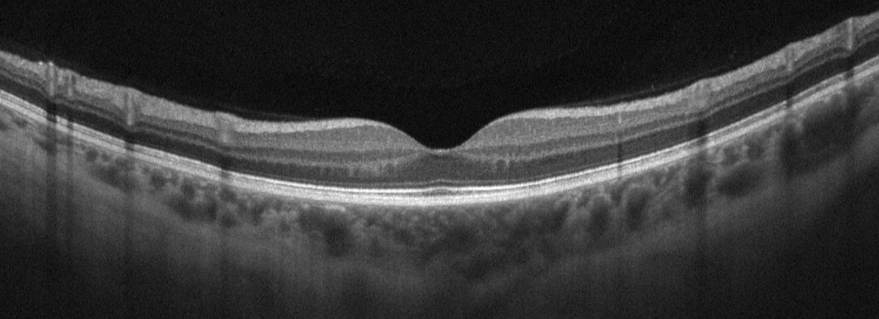 Impression: no evidence of AMD, DME, ERM, RAO, RVO, or VID.